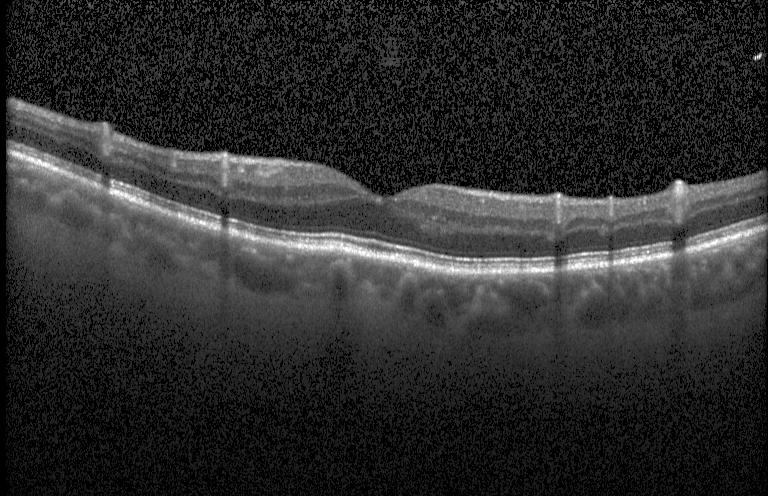
Impression: neither choroidal neovascularization, diabetic macular edema, nor drusen.